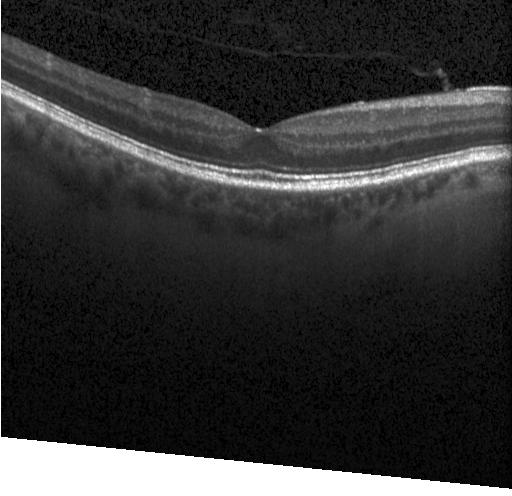
Optical coherence tomography scan. Dx: no CNV, DME, or drusen.